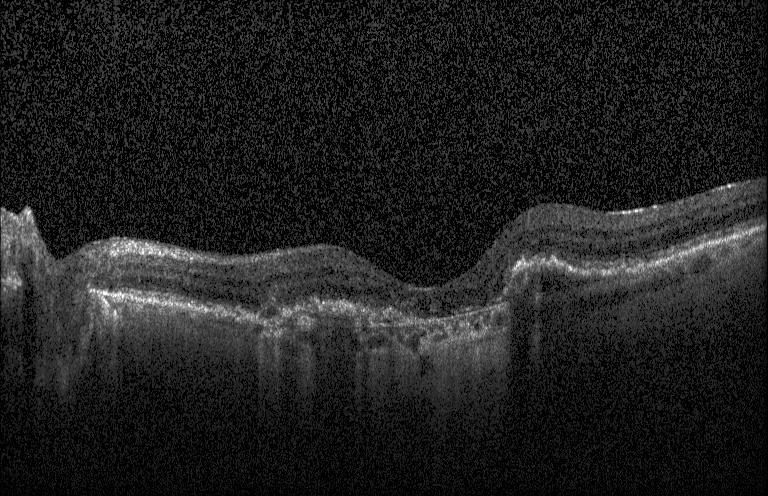 Optical coherence tomography B-scan.
Finding: a choroidal neovascular membrane.